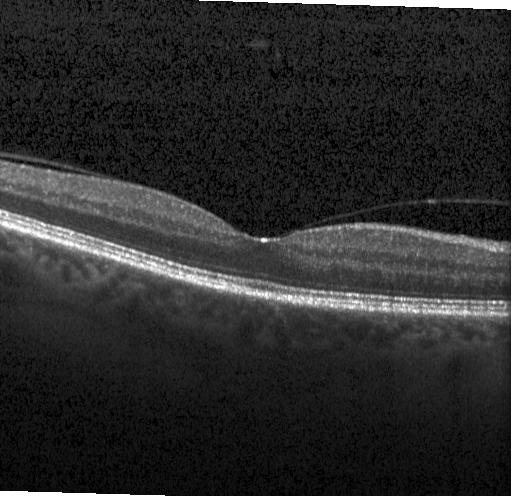

OCT finding: no choroidal neovascularization, diabetic macular edema, or drusen.